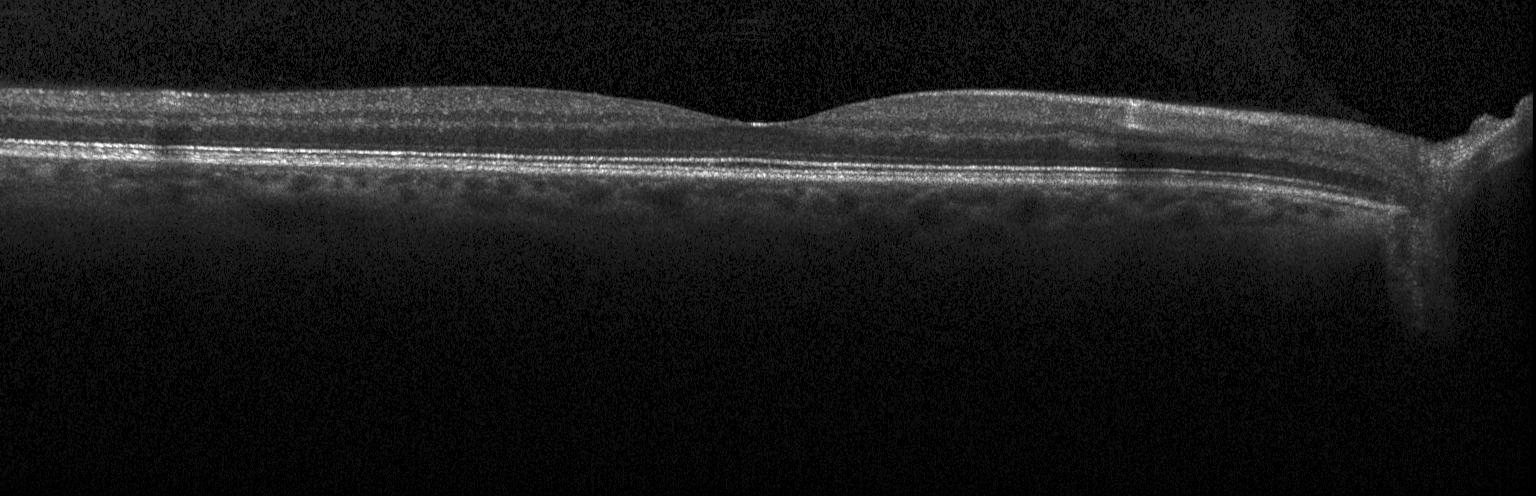
Acquired on a Heidelberg Spectralis, SD-OCT, optical coherence tomography scan — Finding: neither CNV, DME, nor drusen.